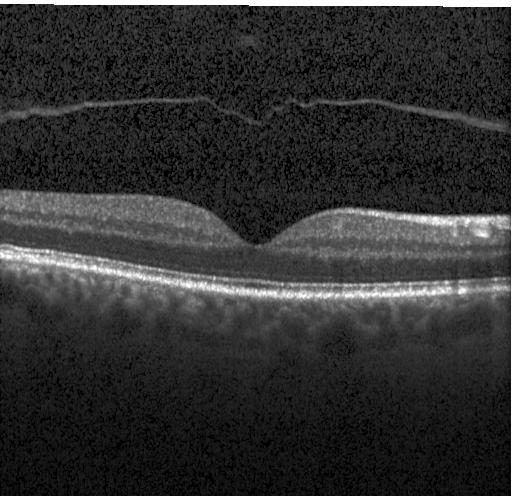 Macular OCT: neither choroidal neovascularization, diabetic macular edema, nor drusen.